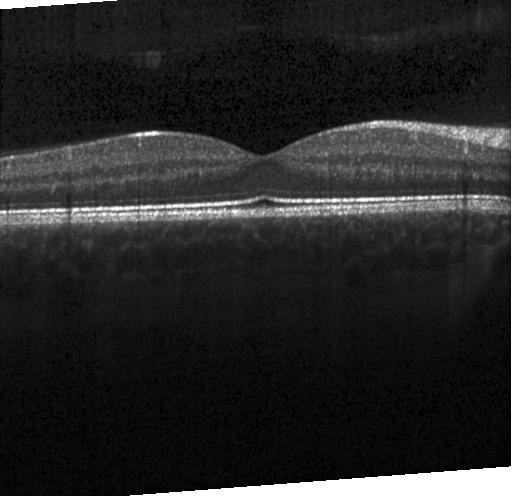

Instrument: Heidelberg Spectralis, spectral-domain OCT, OCT line scan, macular scan
Dx: no CNV, DME, or drusen.